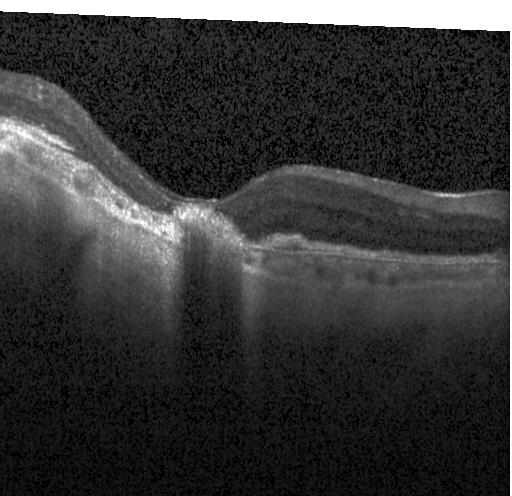 Assessment: choroidal neovascularization (CNV).